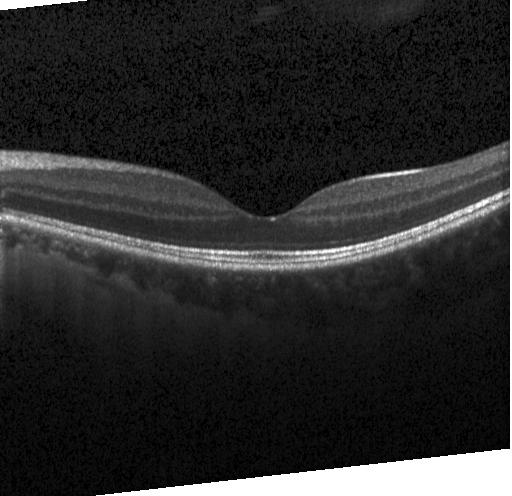

Diagnosis: no choroidal neovascularization, diabetic macular edema, or drusen.